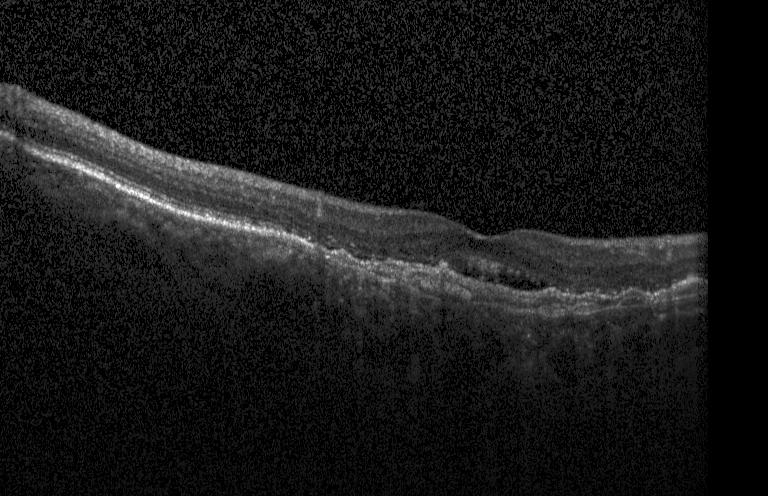
Spectral-domain optical coherence tomography. Fovea-centered. Acquired on a Heidelberg Spectralis. Retinal OCT B-scan.
Assessment: choroidal neovascularization (CNV).